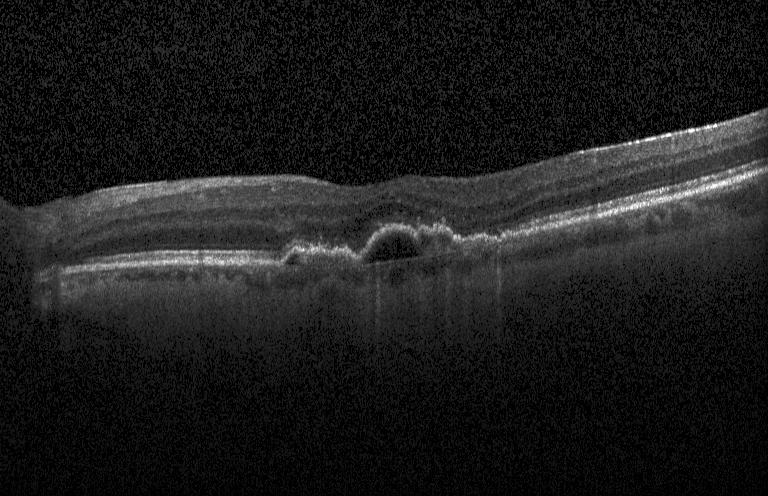 OCT B-scan showing a choroidal neovascular membrane.